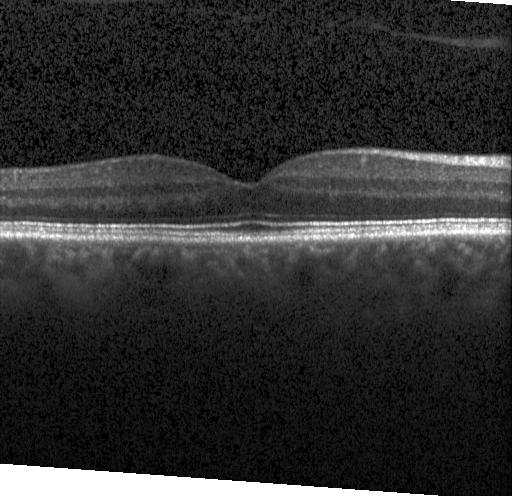

Optical coherence tomography scan.
Dx: no choroidal neovascularization, no diabetic macular edema, and no drusen.